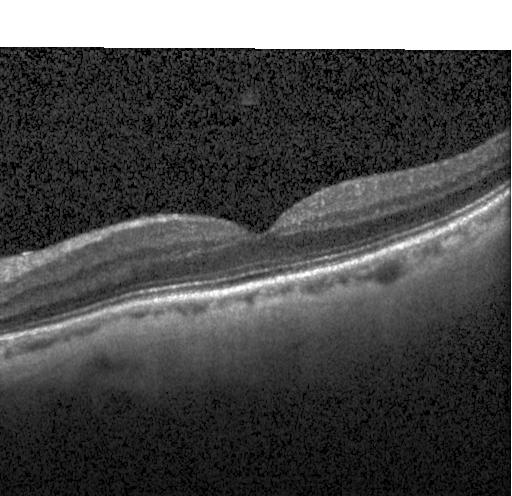
Optical coherence tomography B-scan
OCT finding: no CNV, no DME, and no drusen.